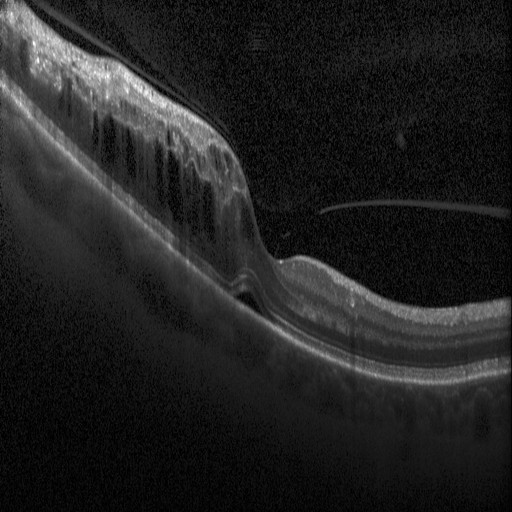 Retinal OCT cross-section.
Impression: diabetic macular edema.